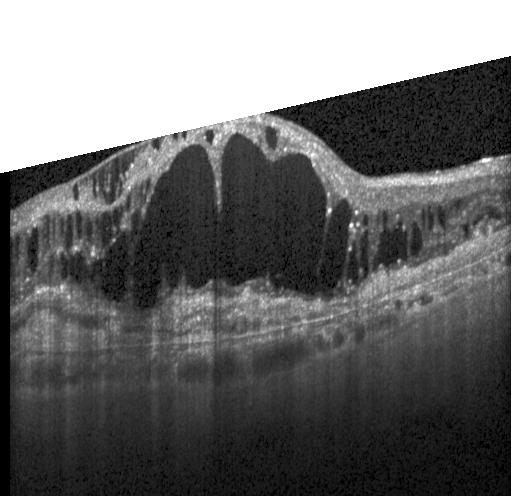
Finding: choroidal neovascularization.